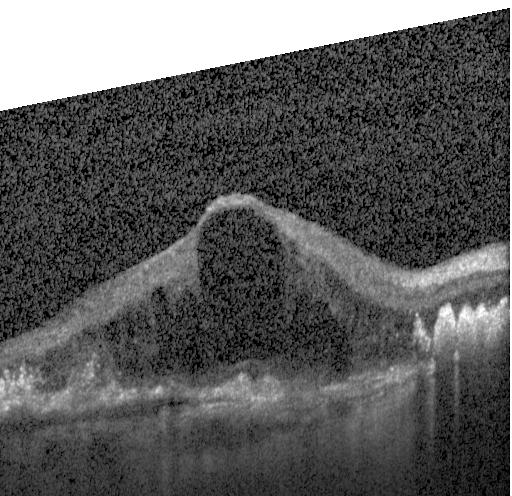
Retinal OCT B-scan.
Assessment: CNV.